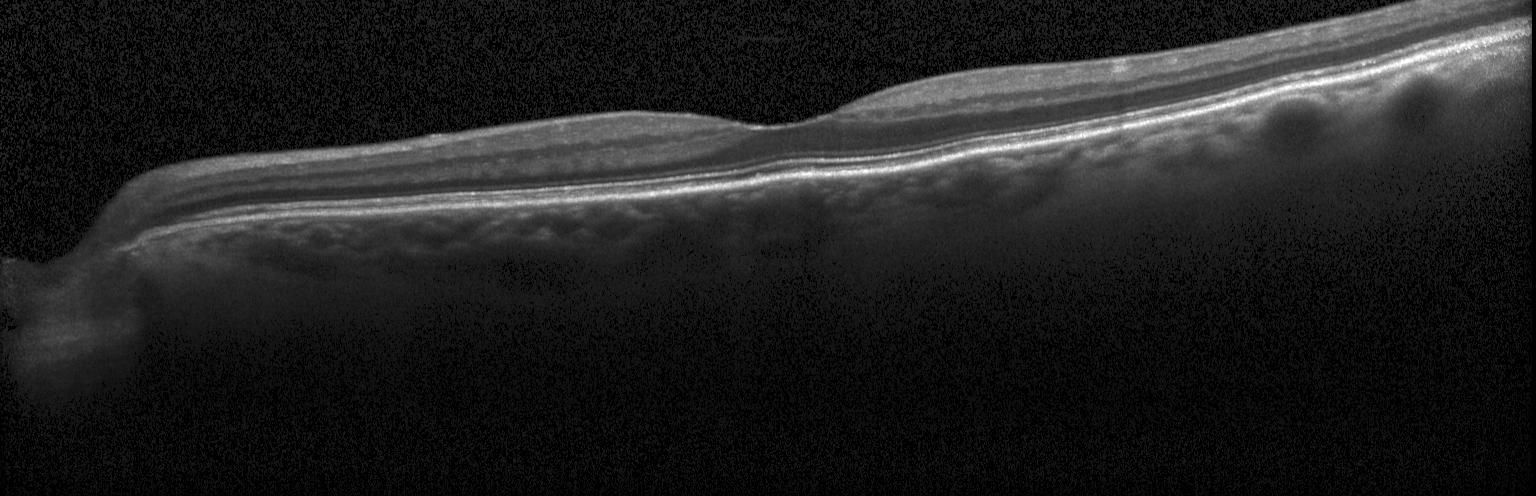
OCT finding: neither choroidal neovascularization, diabetic macular edema, nor drusen.